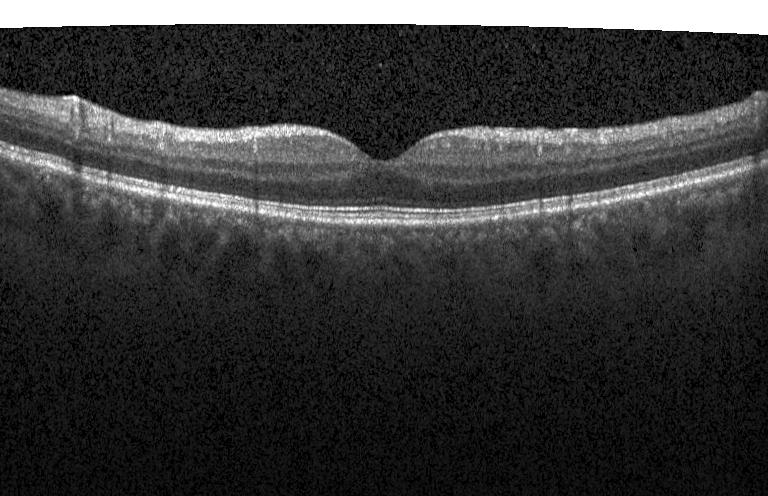

No evidence of choroidal neovascularization, diabetic macular edema, or drusen.